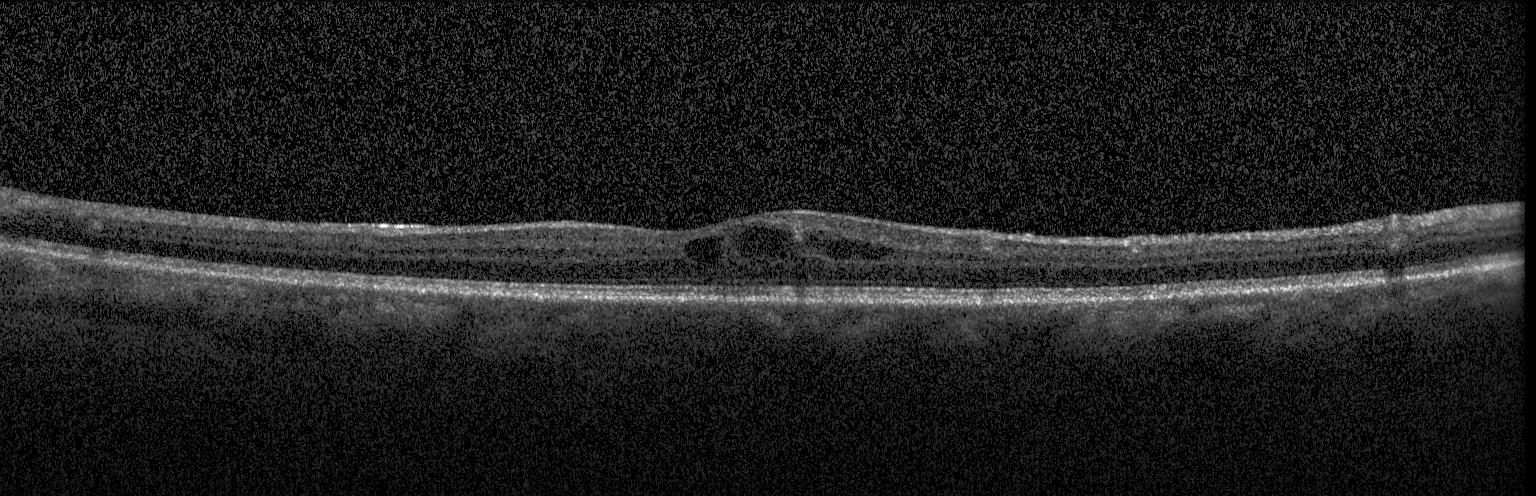

Spectral-domain OCT B-scan: diabetic macular edema.